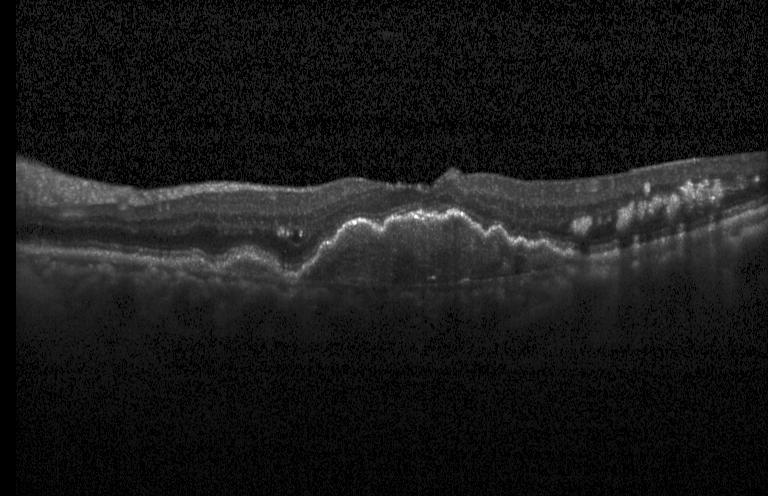
Retinal OCT B-scan
Diagnosis: a choroidal neovascular membrane.